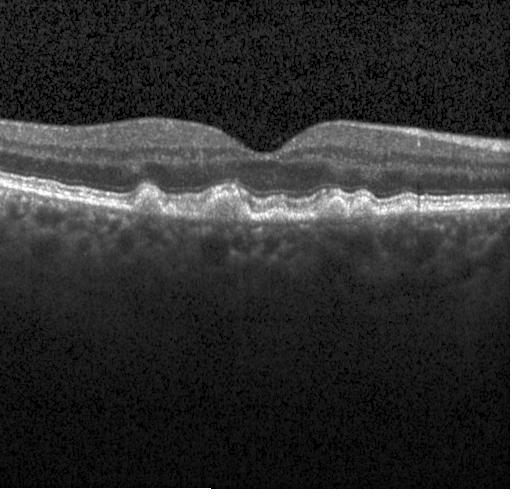

Spectral-domain OCT, acquired on a Heidelberg Spectralis, horizontal scan through the fovea, OCT B-scan — Diagnosis: multiple drusen.